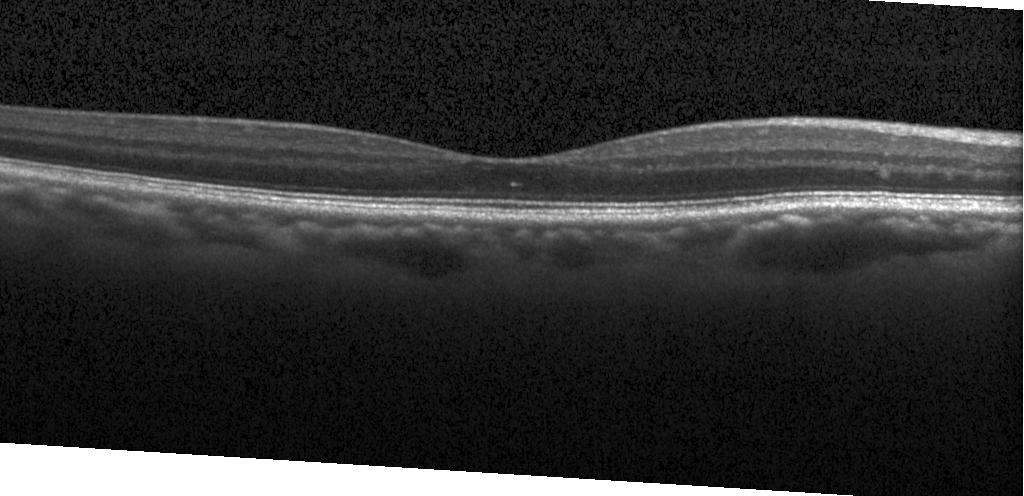 Dx: no CNV, DME, or drusen.